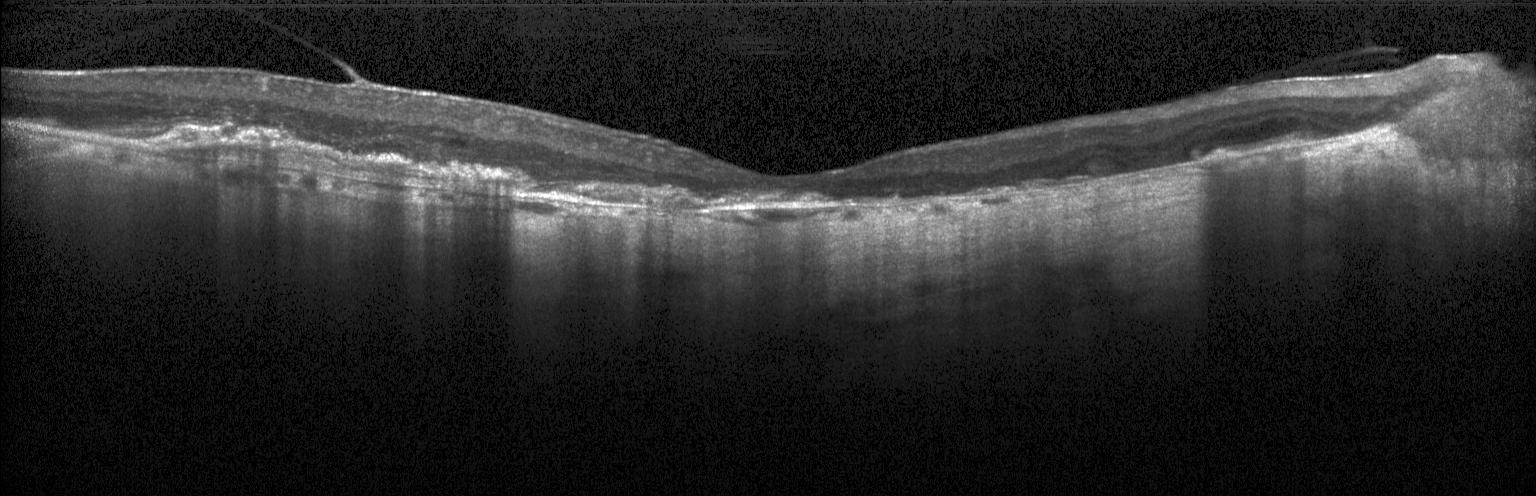
Heidelberg Spectralis OCT system; retinal OCT B-scan; spectral-domain OCT.
OCT finding: CNV.